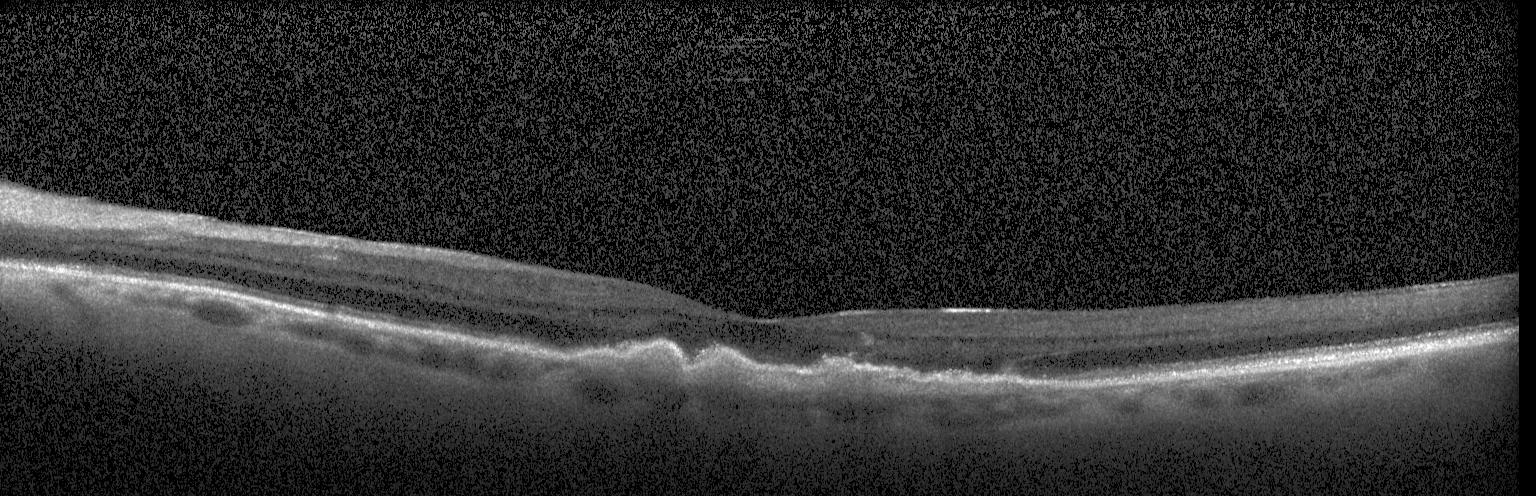 OCT B-scan. Centered on the fovea. Spectral-domain OCT. Acquired on a Heidelberg Spectralis.
Dx: drusen.